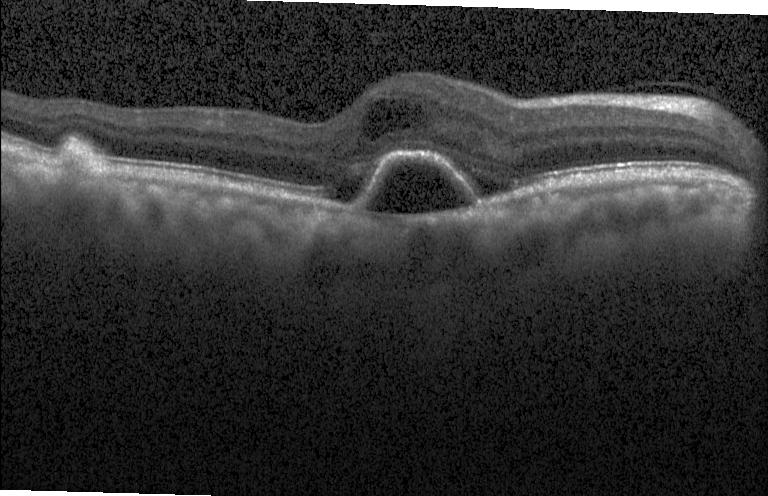

Optical coherence tomography scan — Impression: a choroidal neovascular membrane.